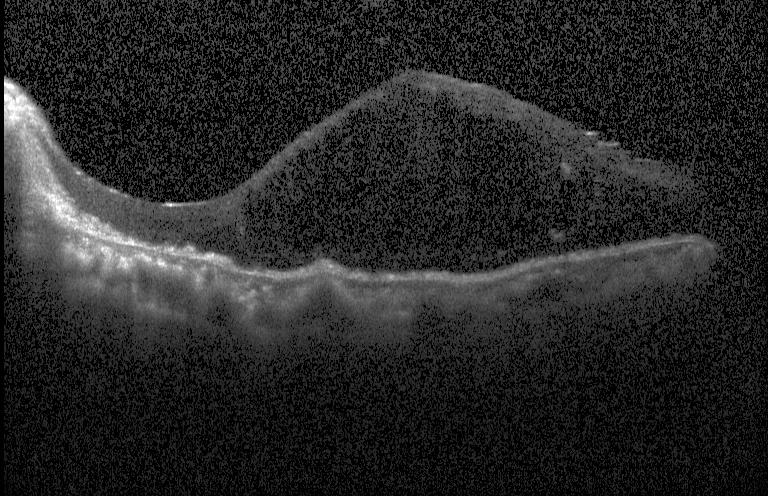 Diagnosis: diabetic macular edema (DME).